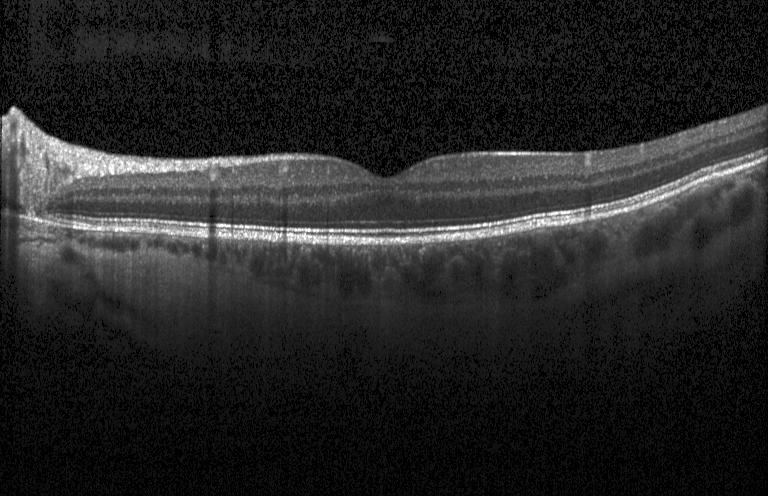

Macular OCT: no evidence of choroidal neovascularization, diabetic macular edema, or drusen.